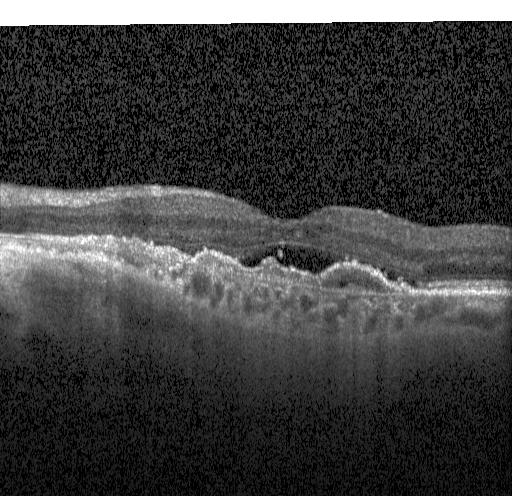
Retinal OCT B-scan · Heidelberg Spectralis OCT system. Macular OCT: a choroidal neovascular membrane.